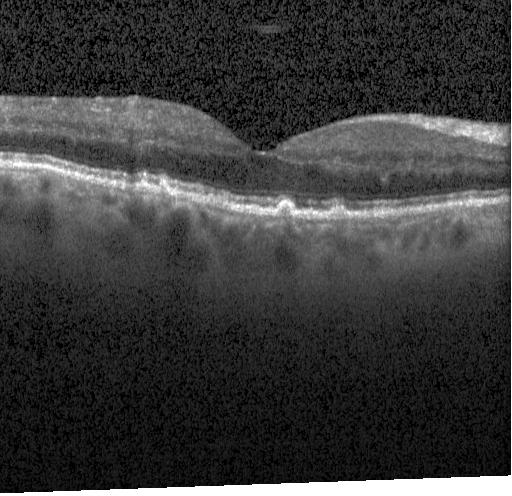
Diagnosis: sub-RPE drusenoid deposits.